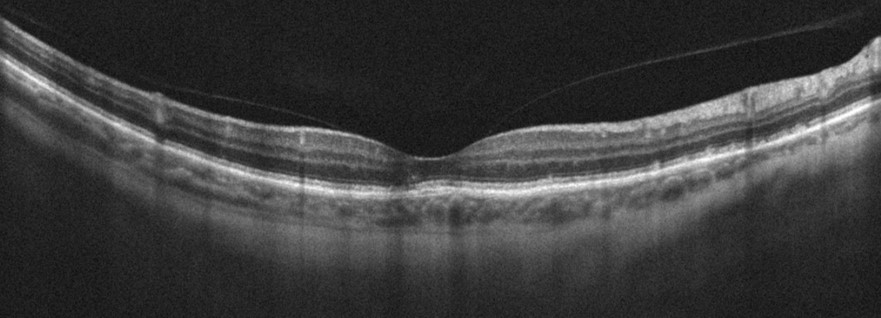
Diagnosis: AMD.